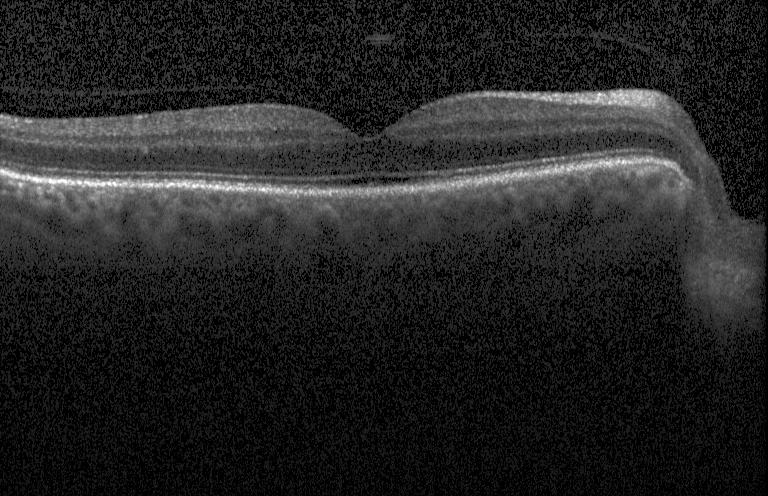 Retinal OCT cross-section showing no evidence of choroidal neovascularization, diabetic macular edema, or drusen.